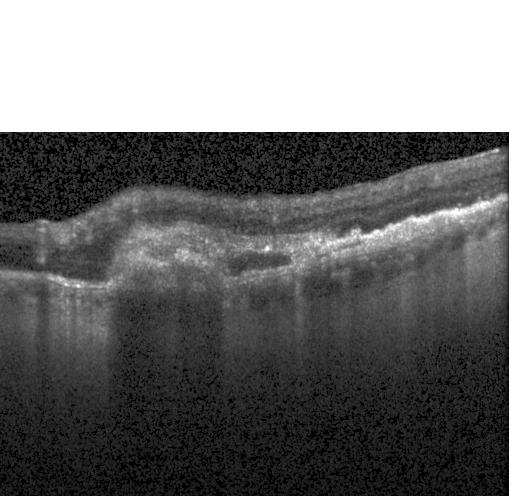
Optical coherence tomography B-scan
The scan shows a choroidal neovascular membrane.